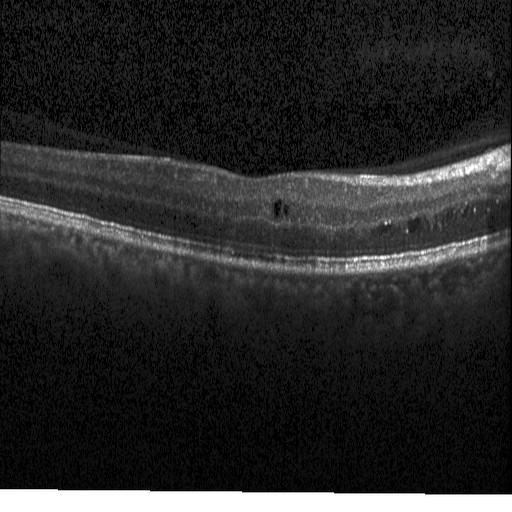 Through the macula · SD-OCT · optical coherence tomography scan — Macular OCT: DME.